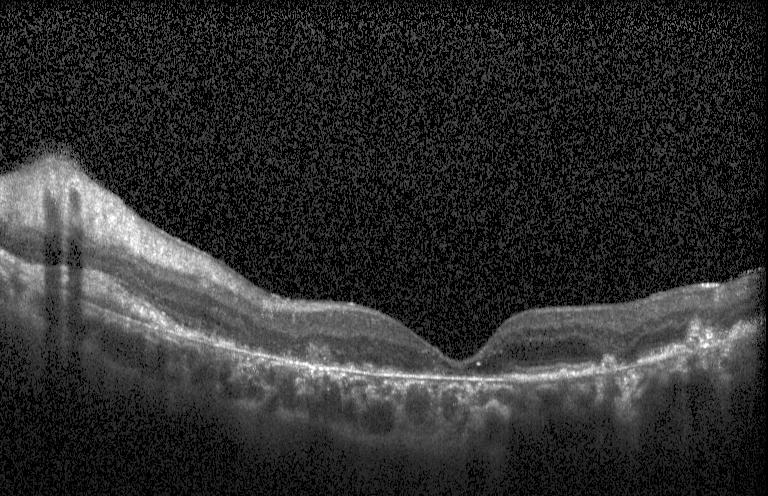
Finding: a choroidal neovascular membrane.